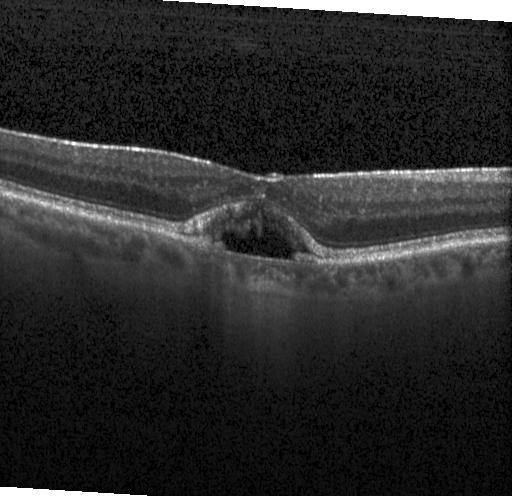 Diagnosis: CNV.